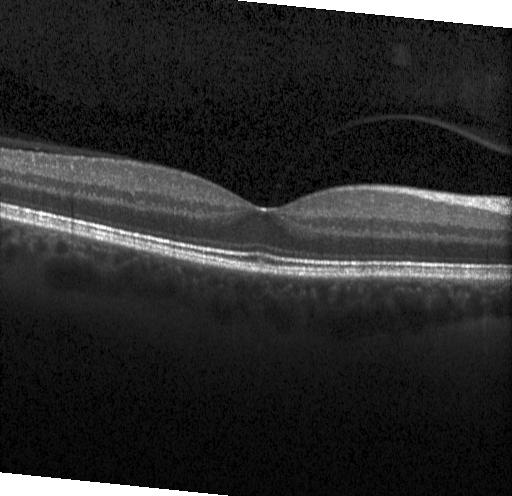

OCT B-scan; Heidelberg Spectralis.
Finding: no evidence of CNV, DME, or drusen.